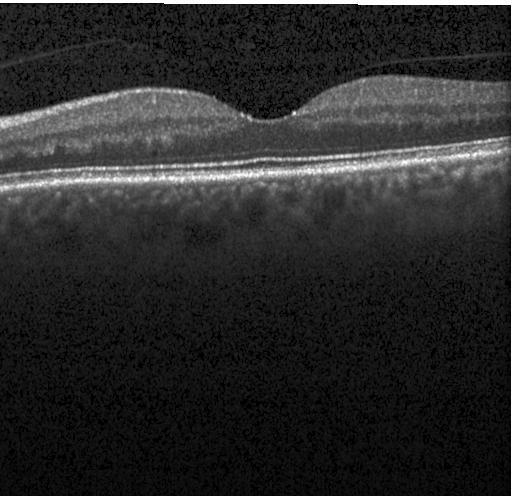
No choroidal neovascularization, diabetic macular edema, or drusen.